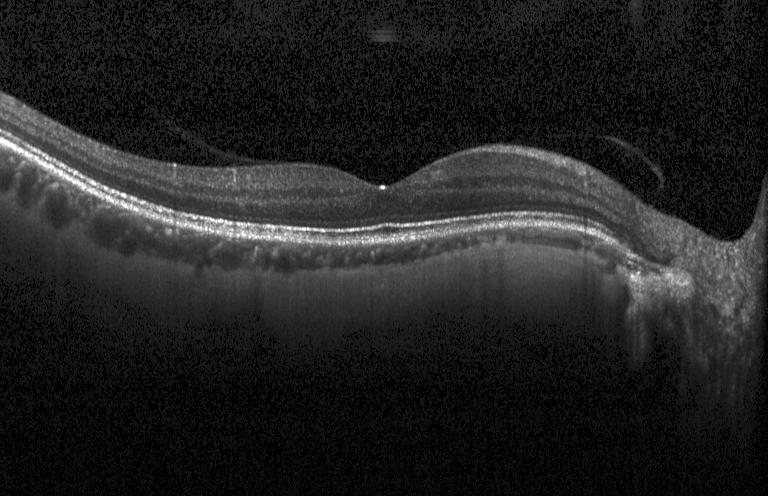

SD-OCT; acquired on a Heidelberg Spectralis; optical coherence tomography B-scan. The scan shows no evidence of choroidal neovascularization, diabetic macular edema, or drusen.